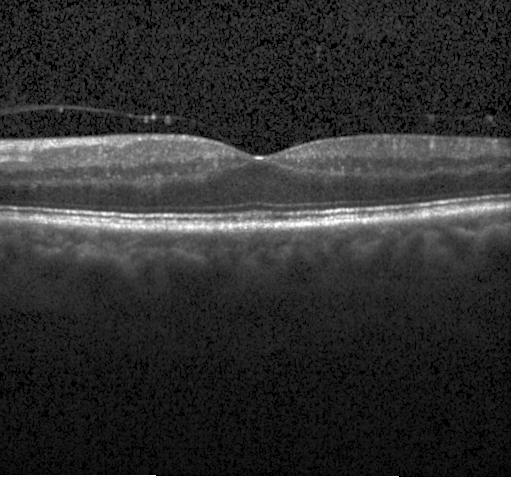
Optical coherence tomography B-scan. Spectral-domain OCT — This B-scan demonstrates no CNV, DME, or drusen.